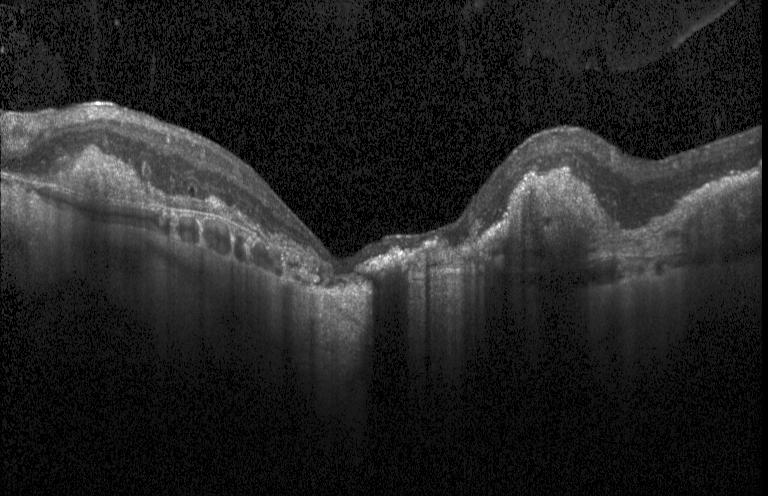

Finding: a choroidal neovascular membrane.